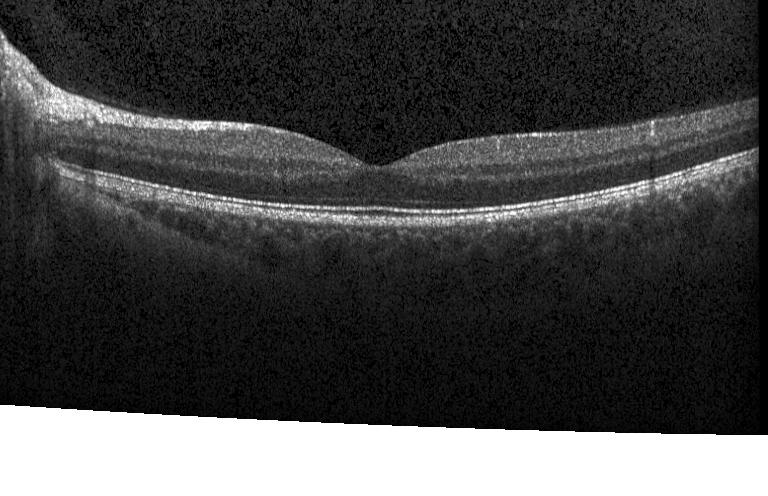 Optical coherence tomography B-scan; spectral-domain optical coherence tomography; through the macula
Assessment: no choroidal neovascularization, diabetic macular edema, or drusen.